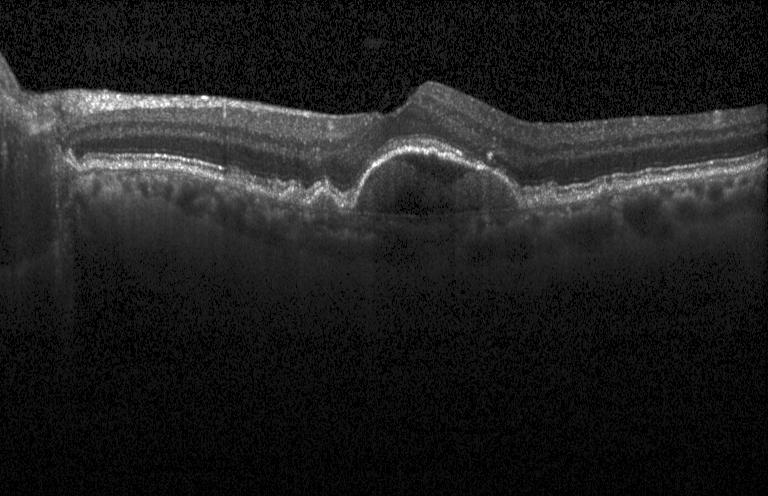
OCT B-scan, Heidelberg Spectralis, through the macula, SD-OCT. Dx: sub-RPE drusenoid deposits.